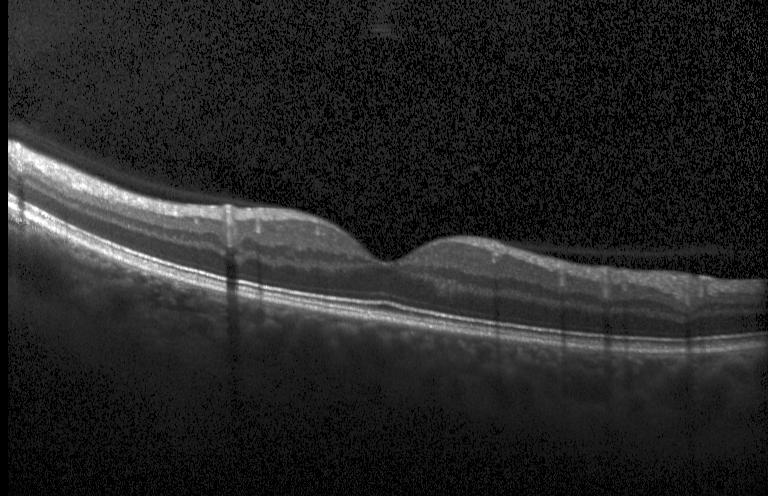

Heidelberg Spectralis. Optical coherence tomography B-scan. Centered on the fovea. SD-OCT.
Dx: no choroidal neovascularization, diabetic macular edema, or drusen.